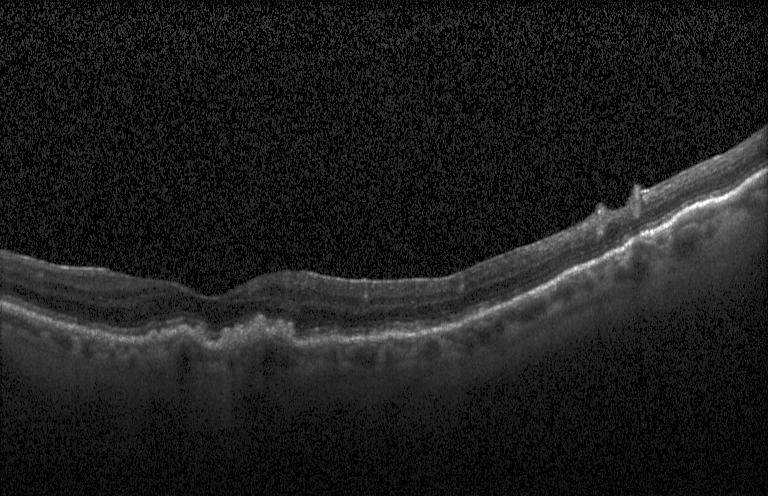 Heidelberg Spectralis OCT system; OCT B-scan; macular scan
The scan shows choroidal neovascularization (CNV).